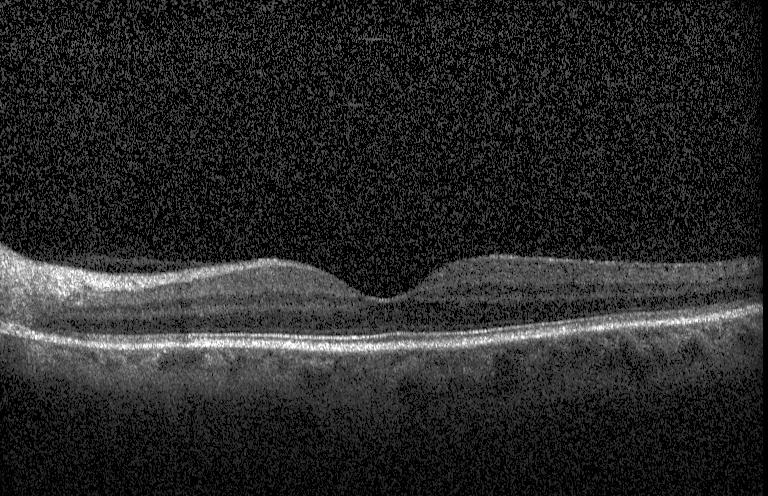

Spectral-domain optical coherence tomography; OCT B-scan; Heidelberg Spectralis
Dx: no evidence of choroidal neovascularization, diabetic macular edema, or drusen.